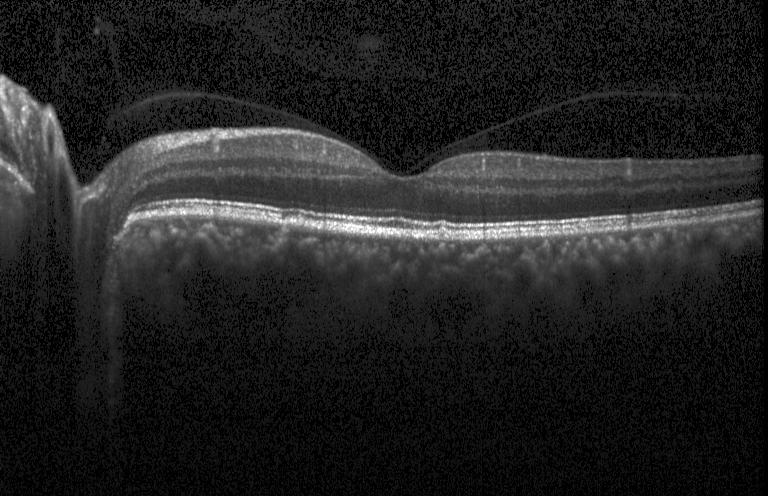

OCT B-scan. Heidelberg Spectralis.
Assessment: multiple drusen.